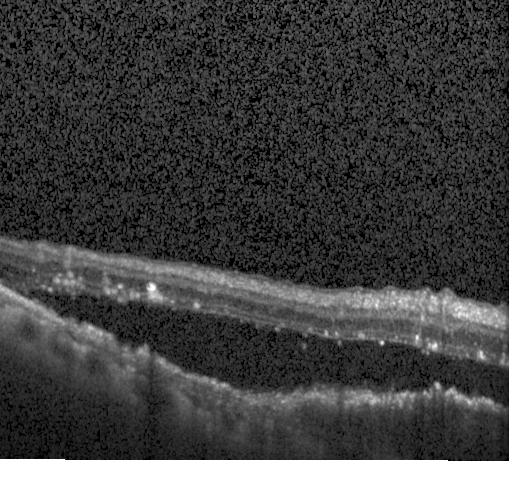
Acquired on a Heidelberg Spectralis, retinal OCT cross-section, spectral-domain optical coherence tomography, horizontal scan through the fovea. Diagnosis: a choroidal neovascular membrane.